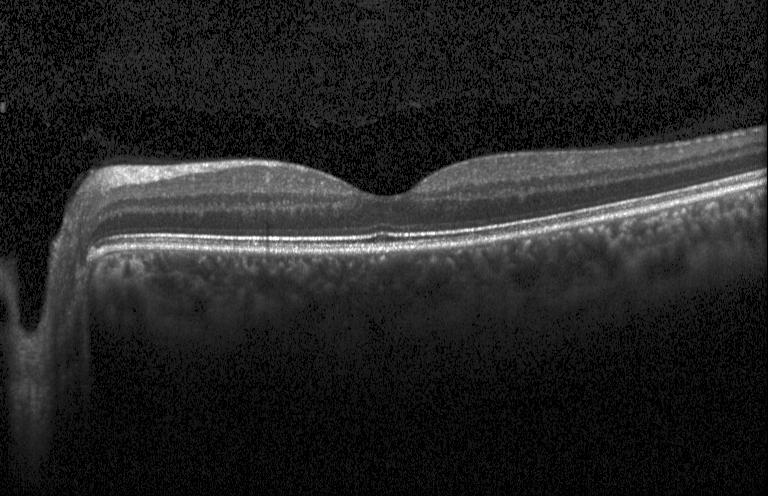

Spectral-domain optical coherence tomography. OCT line scan — Macular OCT: neither choroidal neovascularization, diabetic macular edema, nor drusen.